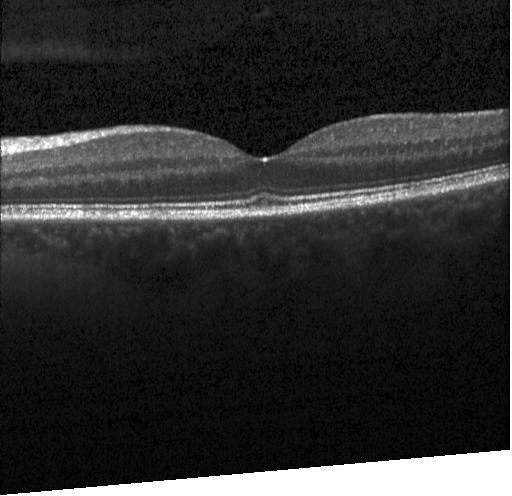

OCT B-scan, SD-OCT.
Diagnosis: no choroidal neovascularization, no diabetic macular edema, and no drusen.